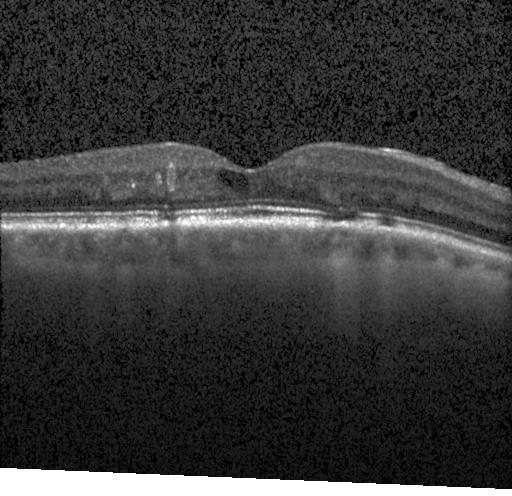

OCT B-scan; Heidelberg Spectralis OCT system. Impression: diabetic macular edema.